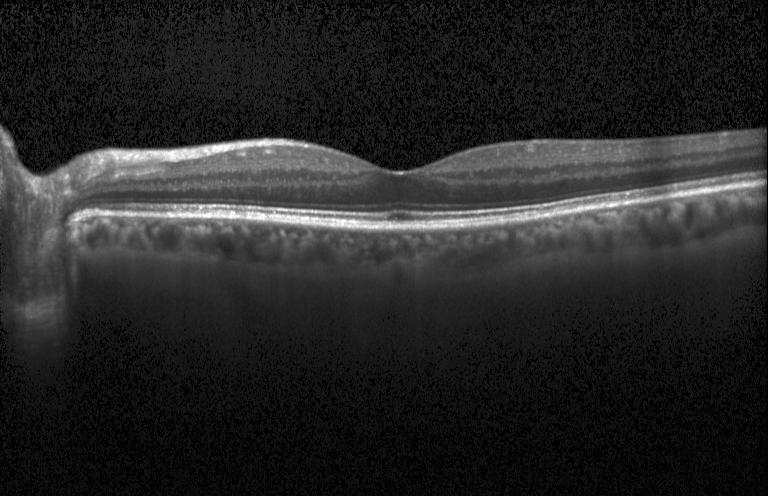

OCT scan showing no choroidal neovascularization, no diabetic macular edema, and no drusen.